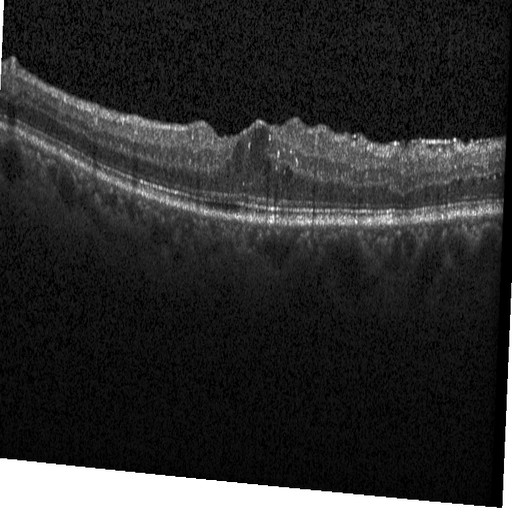 Diagnosis: diabetic macular edema.